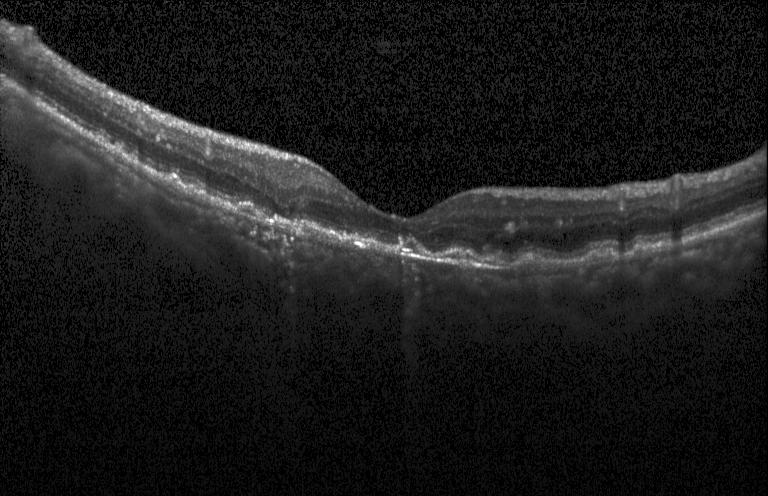

Finding: choroidal neovascularization (CNV).